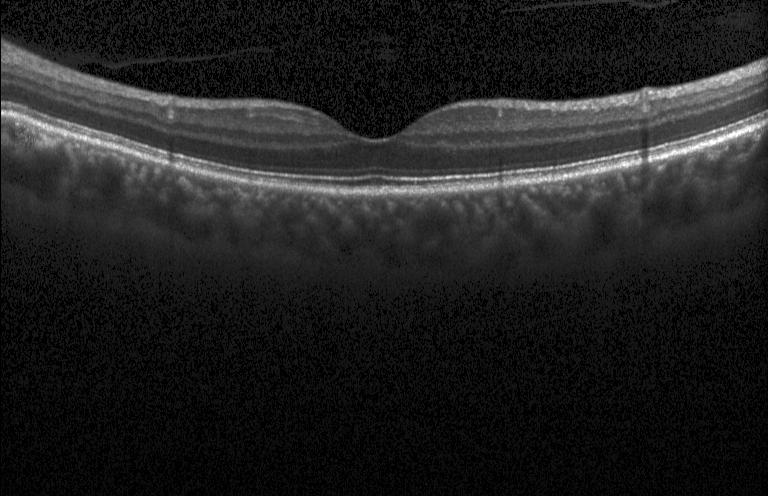
Spectral-domain optical coherence tomography · instrument: Heidelberg Spectralis · OCT B-scan · fovea-centered — OCT finding: no choroidal neovascularization, diabetic macular edema, or drusen.